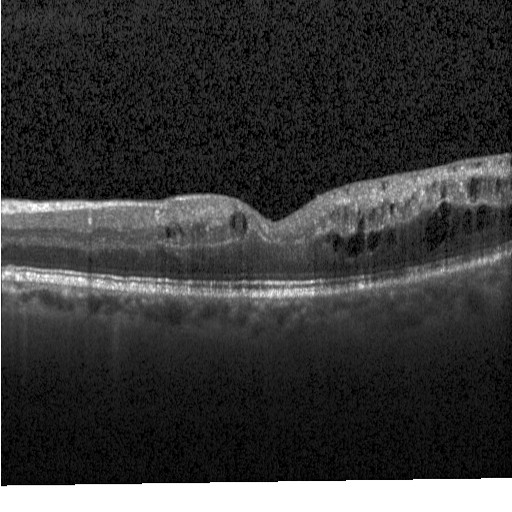
Acquired on a Heidelberg Spectralis. Spectral-domain OCT. Optical coherence tomography scan
Assessment: diabetic macular edema.